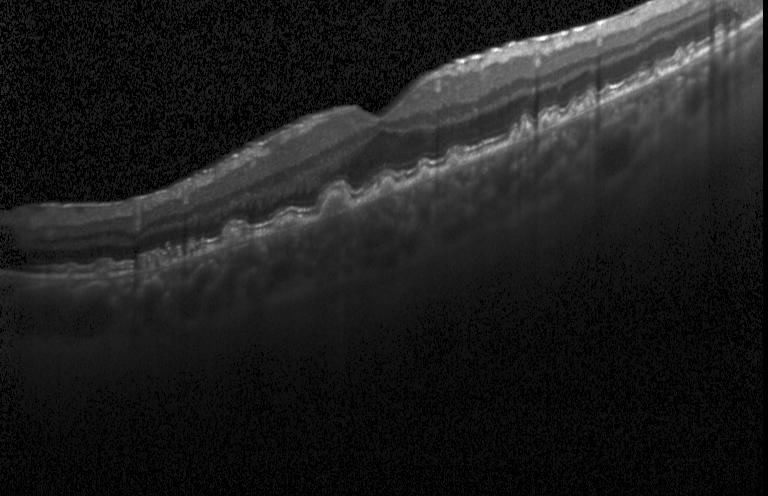

Impression: multiple drusen.